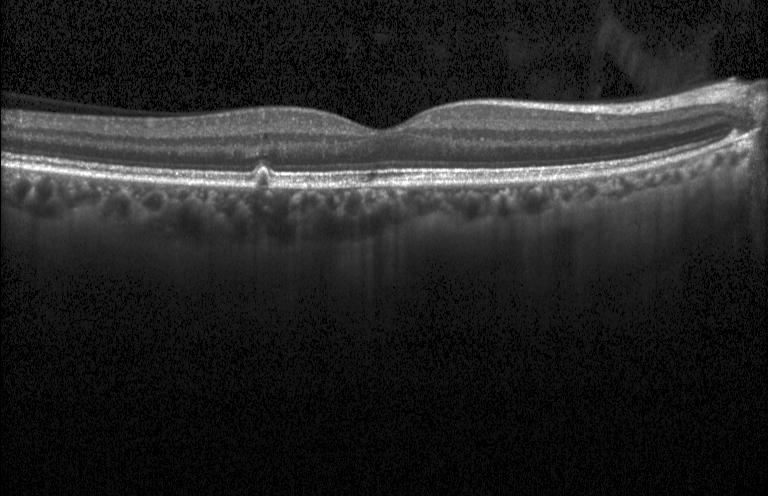

OCT B-scan showing drusen.